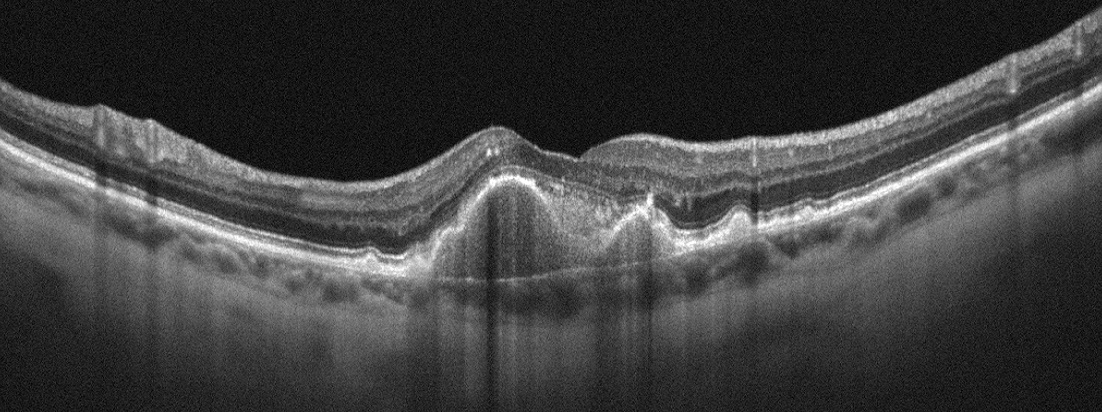

Retinal OCT cross-section, through the macula, acquired on an Optovue Avanti RTVue XR
Dx: AMD.